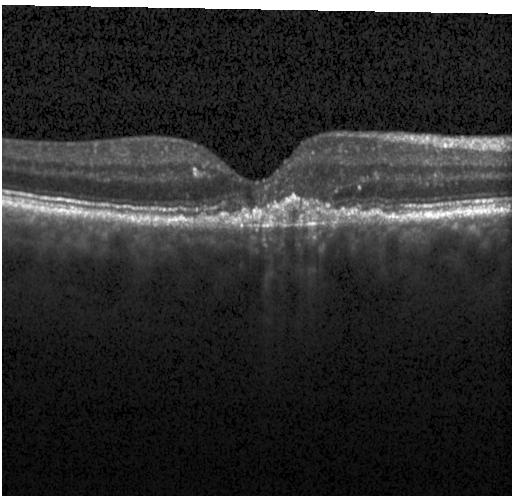

Optical coherence tomography B-scan.
OCT finding: choroidal neovascularization (CNV).